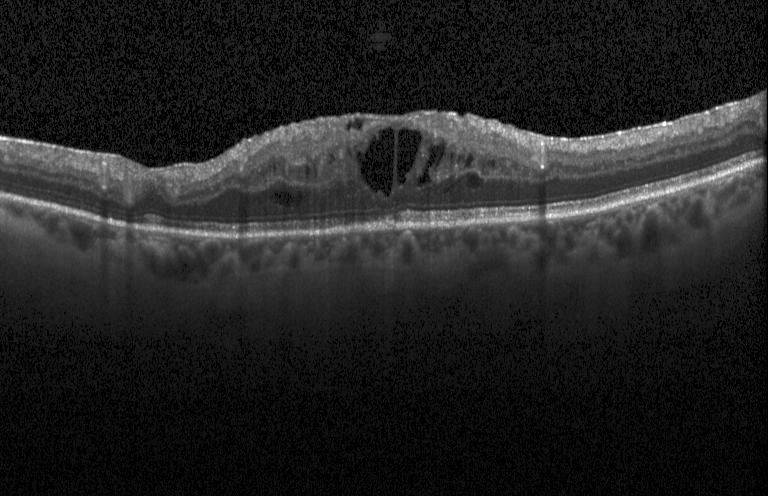
Horizontal scan through the fovea. Heidelberg Spectralis OCT system. OCT B-scan
Assessment: DME.